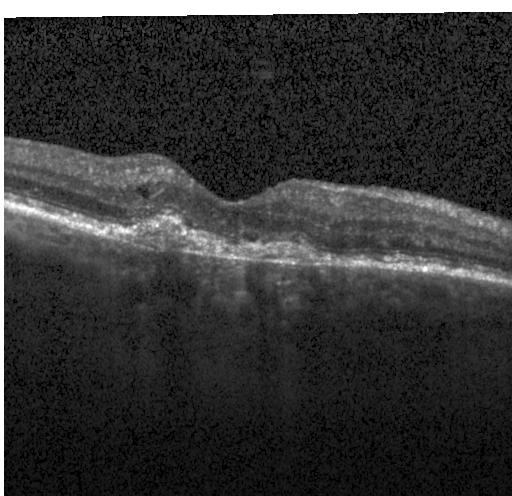

Spectral-domain OCT B-scan: a choroidal neovascular membrane.